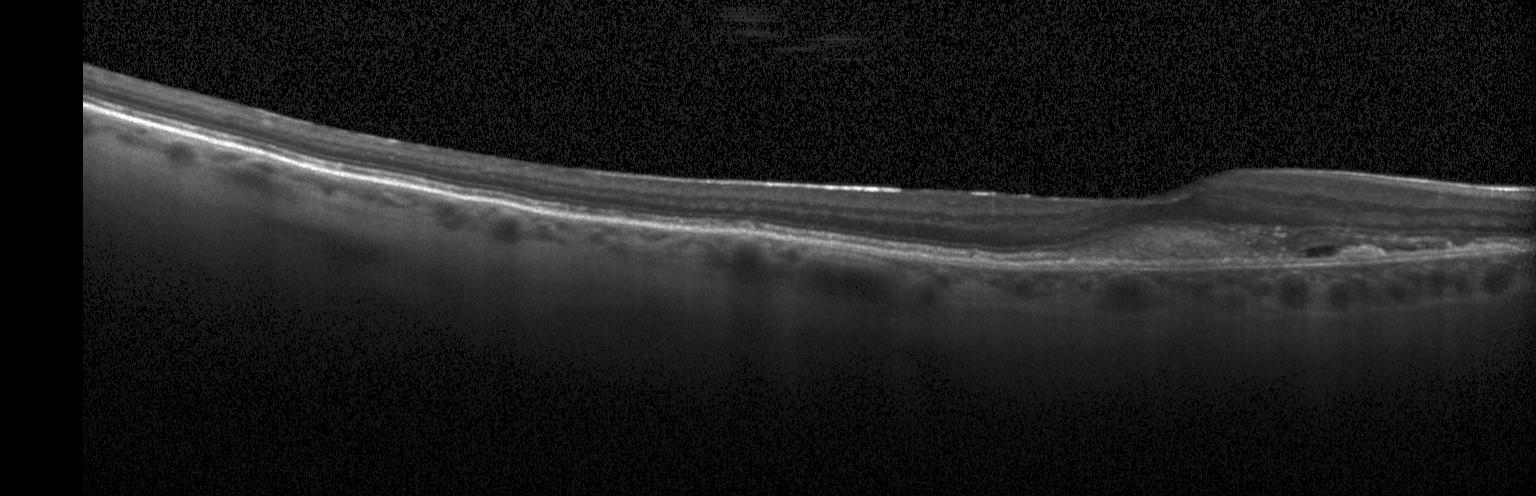
OCT finding: a choroidal neovascular membrane.